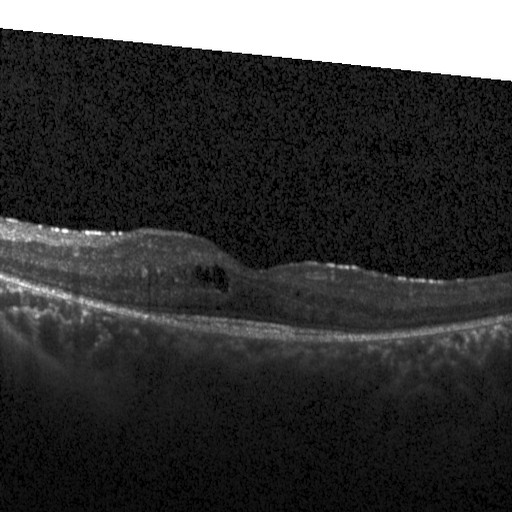
Heidelberg Spectralis. Macular scan. OCT B-scan — The scan shows diabetic macular edema.